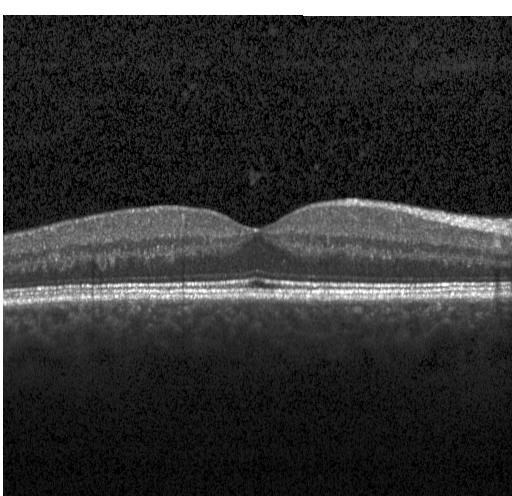 Acquired on a Heidelberg Spectralis; SD-OCT; OCT B-scan; fovea-centered
Finding: no evidence of choroidal neovascularization, diabetic macular edema, or drusen.